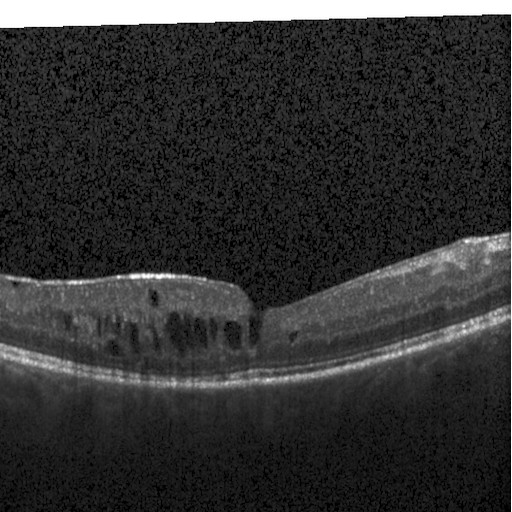
Macular OCT demonstrating diabetic macular edema (DME).